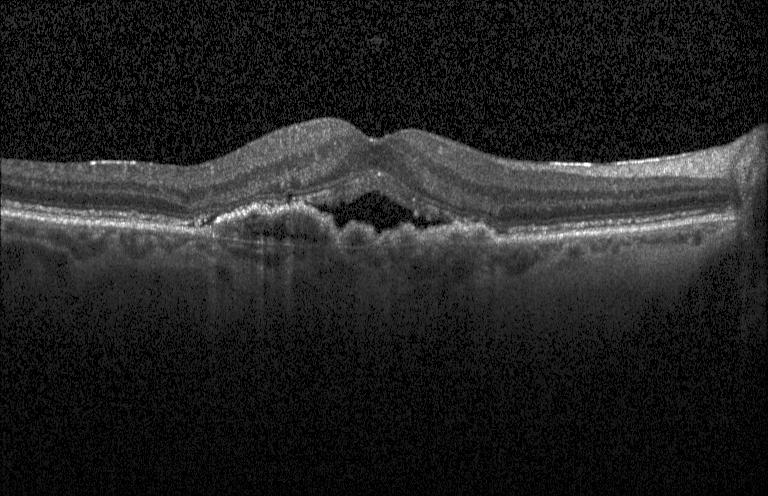

OCT B-scan, centered on the fovea
OCT finding: choroidal neovascularization (CNV).